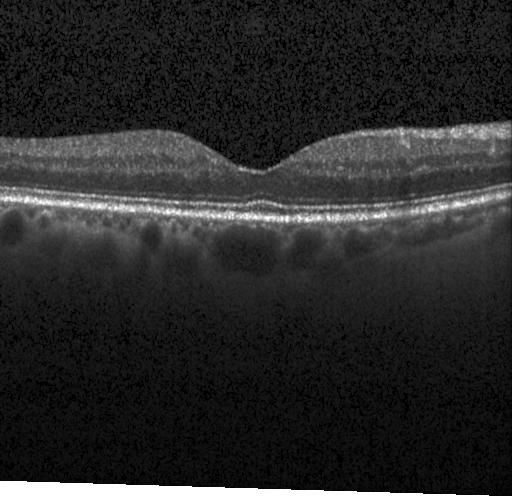 Finding: neither choroidal neovascularization, diabetic macular edema, nor drusen.